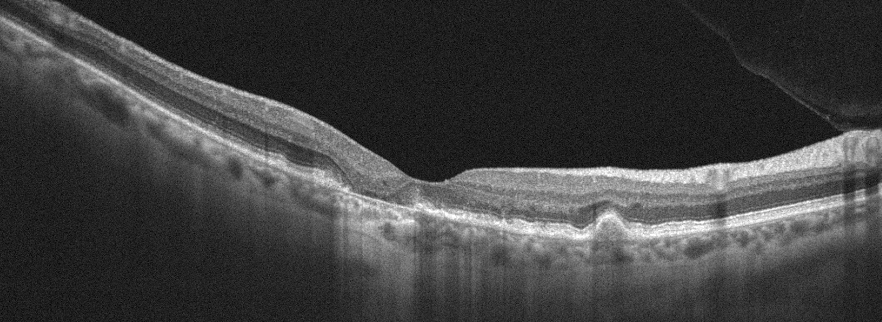 Retinal OCT cross-section — Impression: age-related macular degeneration.